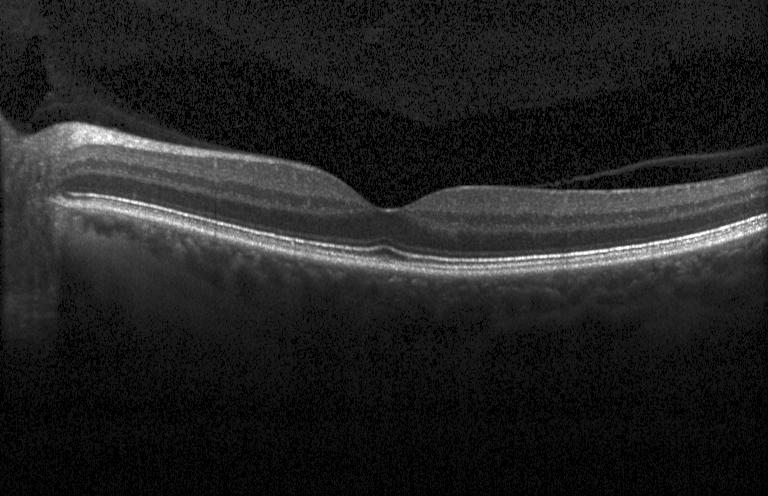 Optical coherence tomography scan. Assessment: no evidence of choroidal neovascularization, diabetic macular edema, or drusen.